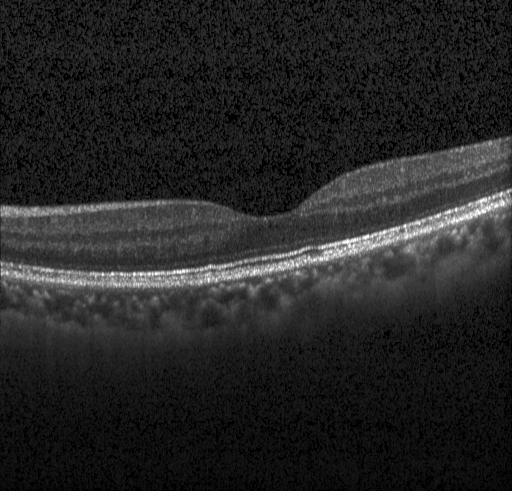 Instrument: Heidelberg Spectralis, spectral-domain OCT, OCT line scan — Diagnosis: no choroidal neovascularization, no diabetic macular edema, and no drusen.